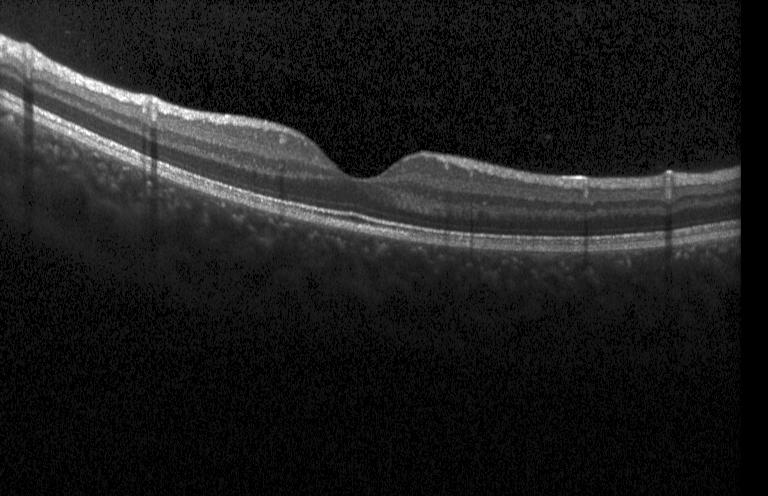 Dx: no evidence of CNV, DME, or drusen.